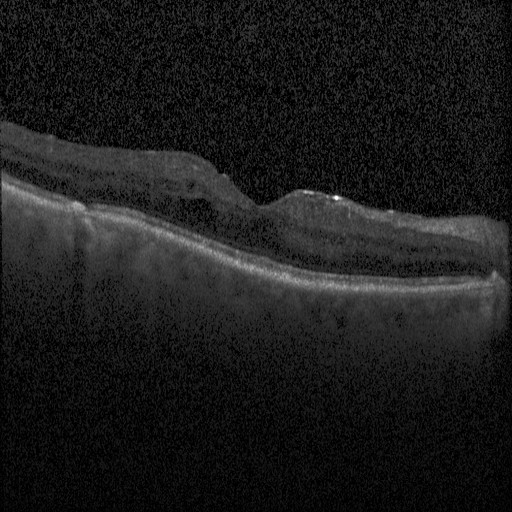
Macular OCT demonstrating diabetic macular edema (DME).